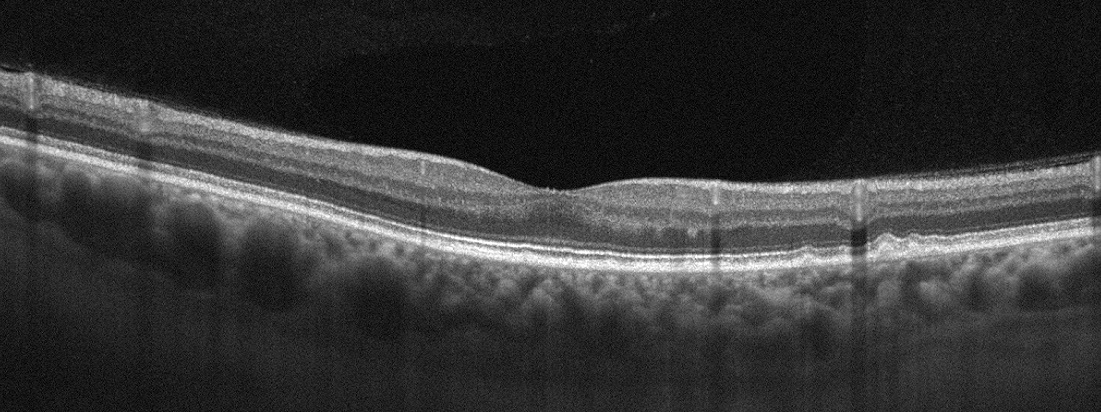

Optical coherence tomography scan — Finding: AMD.